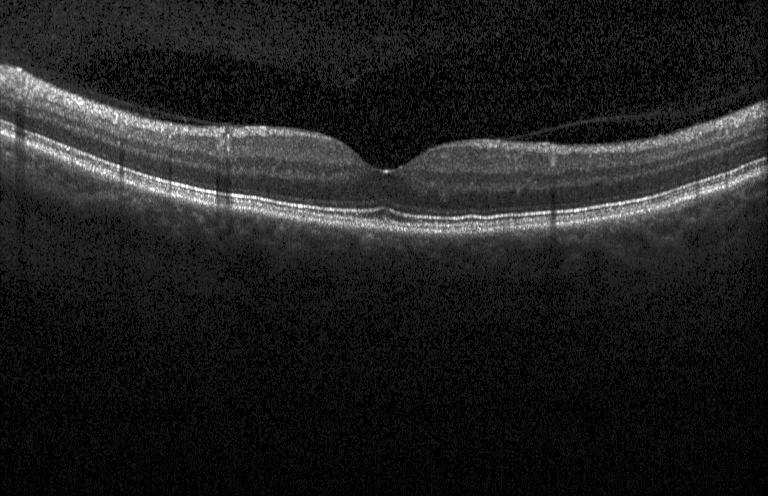 OCT B-scan, spectral-domain optical coherence tomography. Assessment: no CNV, no DME, and no drusen.